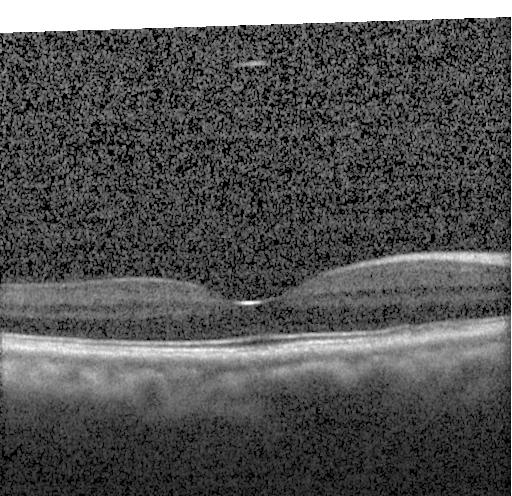 Optical coherence tomography scan
No CNV, DME, or drusen.